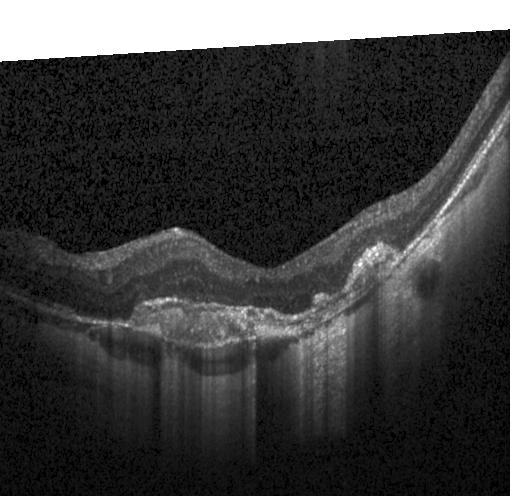

SD-OCT, optical coherence tomography scan, Heidelberg Spectralis. Macular OCT: a choroidal neovascular membrane.